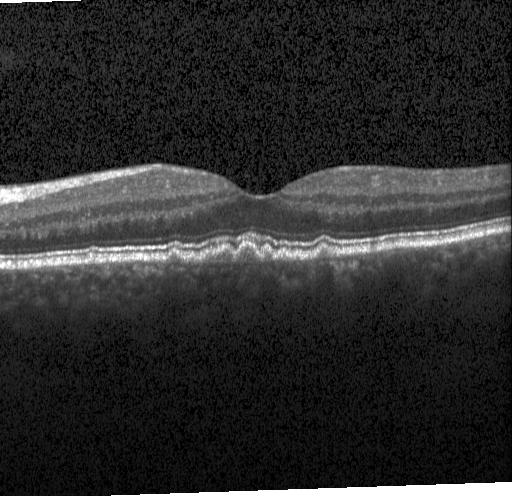
OCT line scan · centered on the fovea.
Impression: drusen.